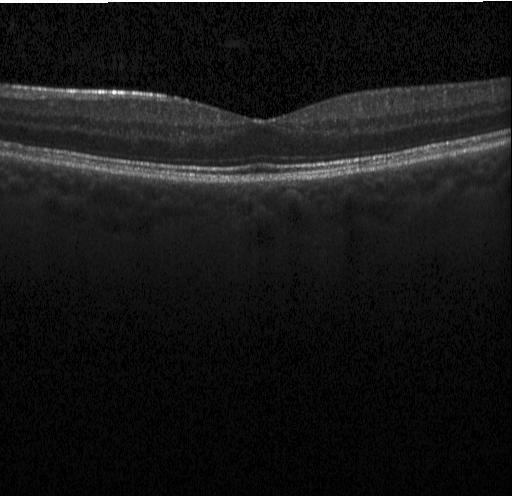
Retinal OCT cross-section.
Diagnosis: no choroidal neovascularization, diabetic macular edema, or drusen.